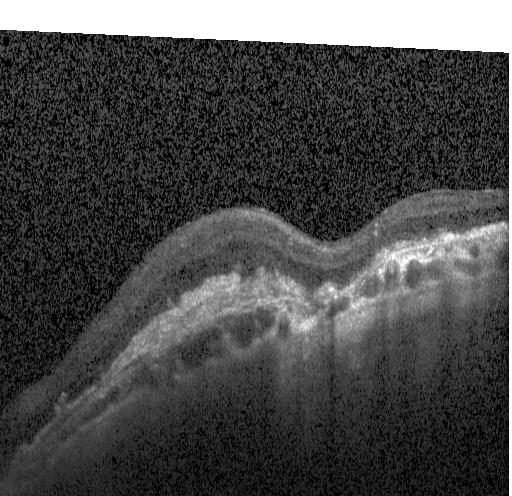
Impression: choroidal neovascularization (CNV).